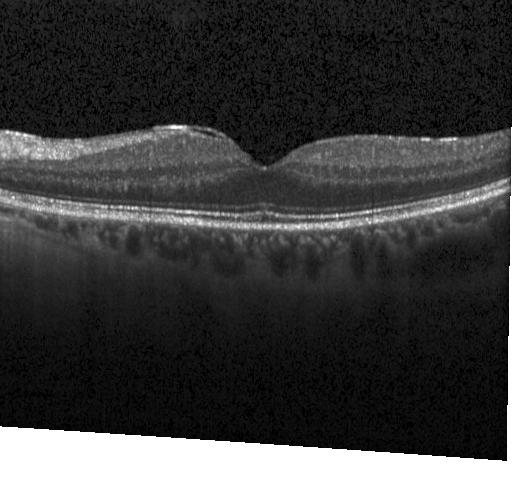 Diagnosis: no CNV, no DME, and no drusen.